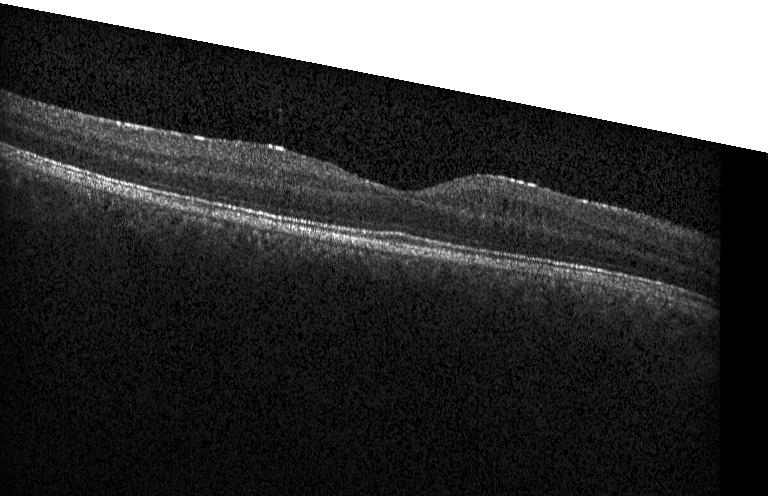

The scan shows DME.